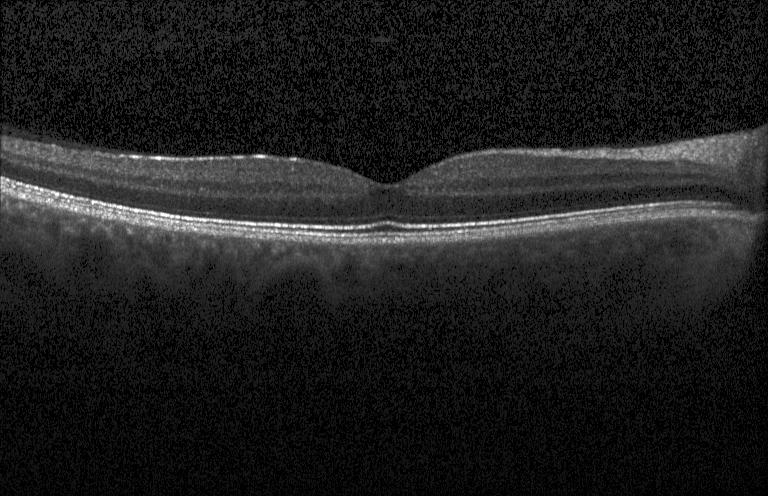
Diagnosis: no choroidal neovascularization, diabetic macular edema, or drusen.